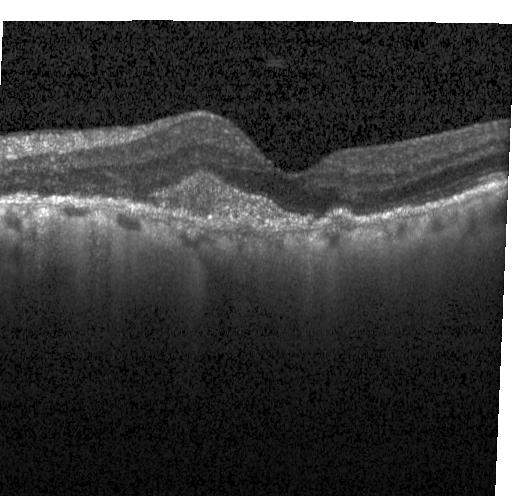

Acquired on a Heidelberg Spectralis. Spectral-domain optical coherence tomography. Retinal OCT B-scan — Dx: CNV.